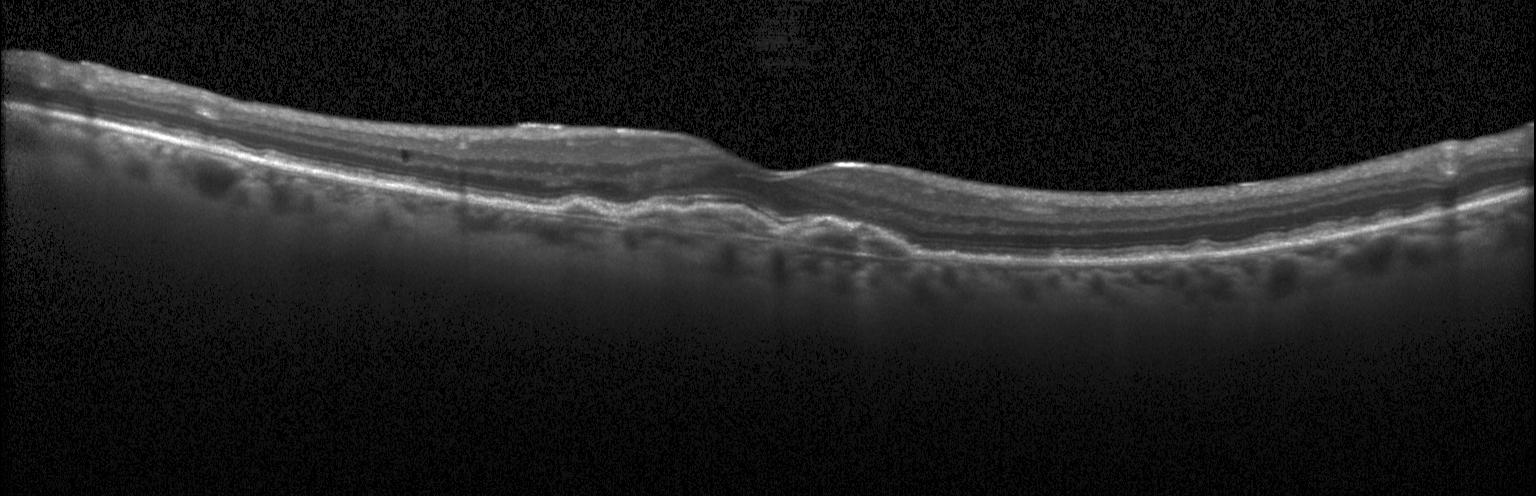 Retinal OCT cross-section
Finding: CNV.